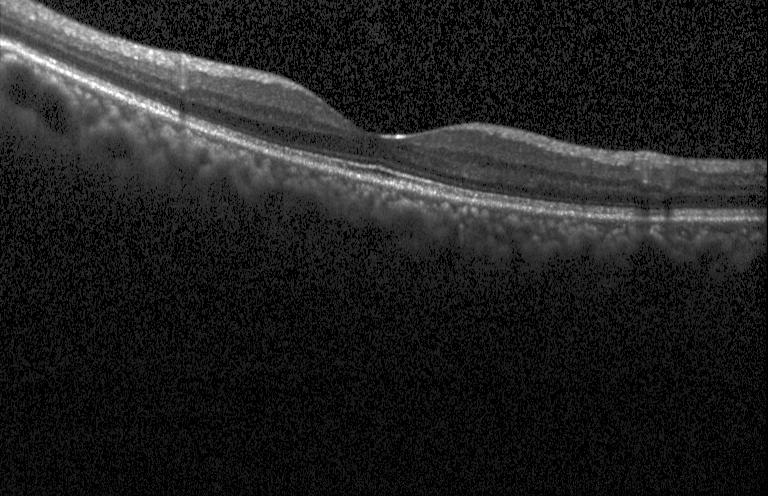 Dx: neither choroidal neovascularization, diabetic macular edema, nor drusen.